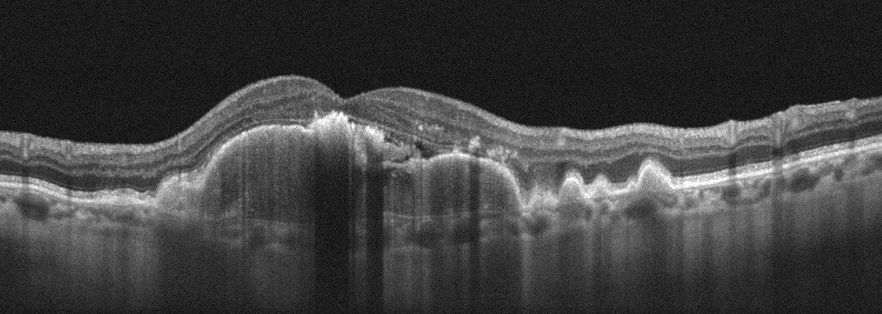 Acquired on an Optovue Avanti RTVue XR. Macular scan. Optical coherence tomography B-scan. Age-related macular degeneration (AMD).